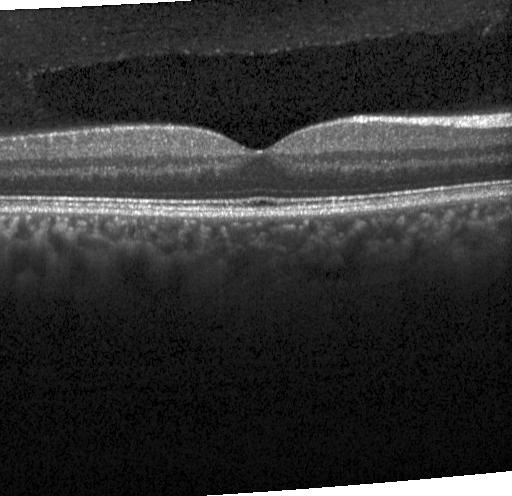 Diagnosis: no evidence of choroidal neovascularization, diabetic macular edema, or drusen.